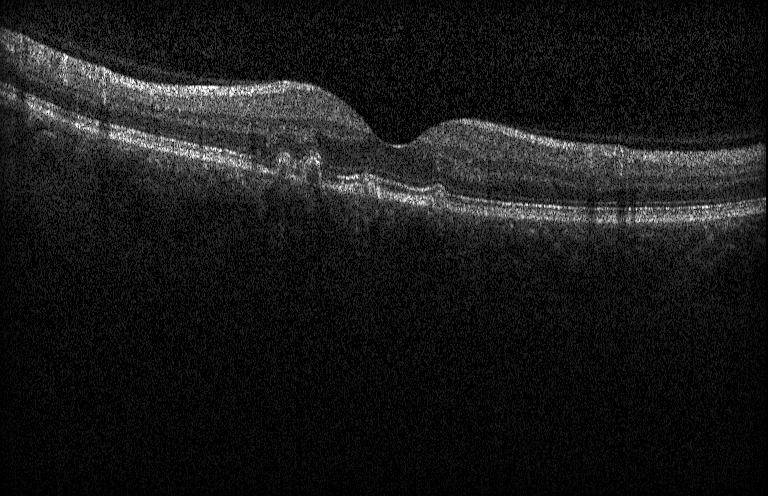 Acquired on a Heidelberg Spectralis; optical coherence tomography B-scan; centered on the fovea; SD-OCT. The scan shows drusen.